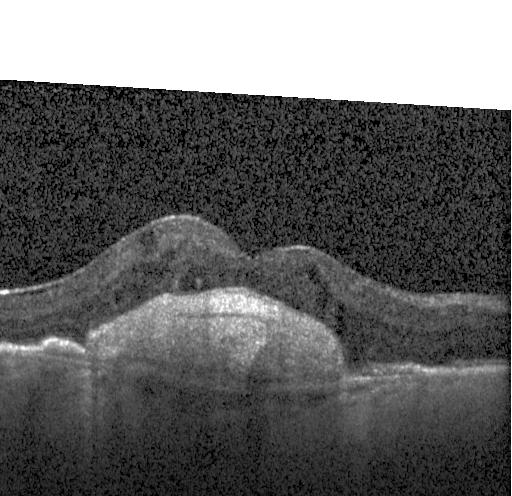 A choroidal neovascular membrane.